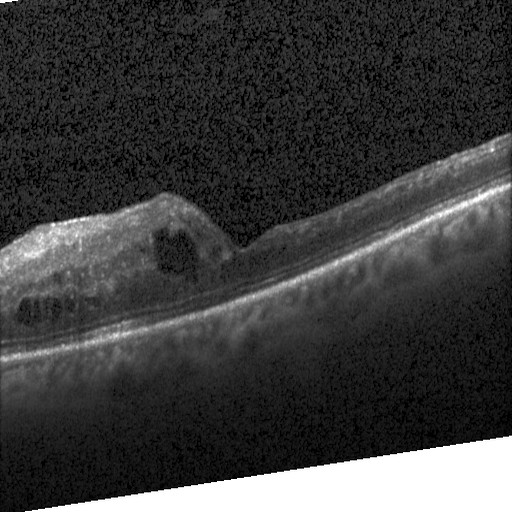 Impression: DME.